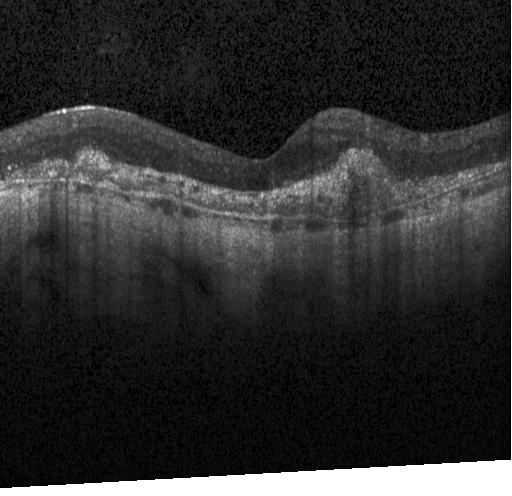 The scan shows a choroidal neovascular membrane.